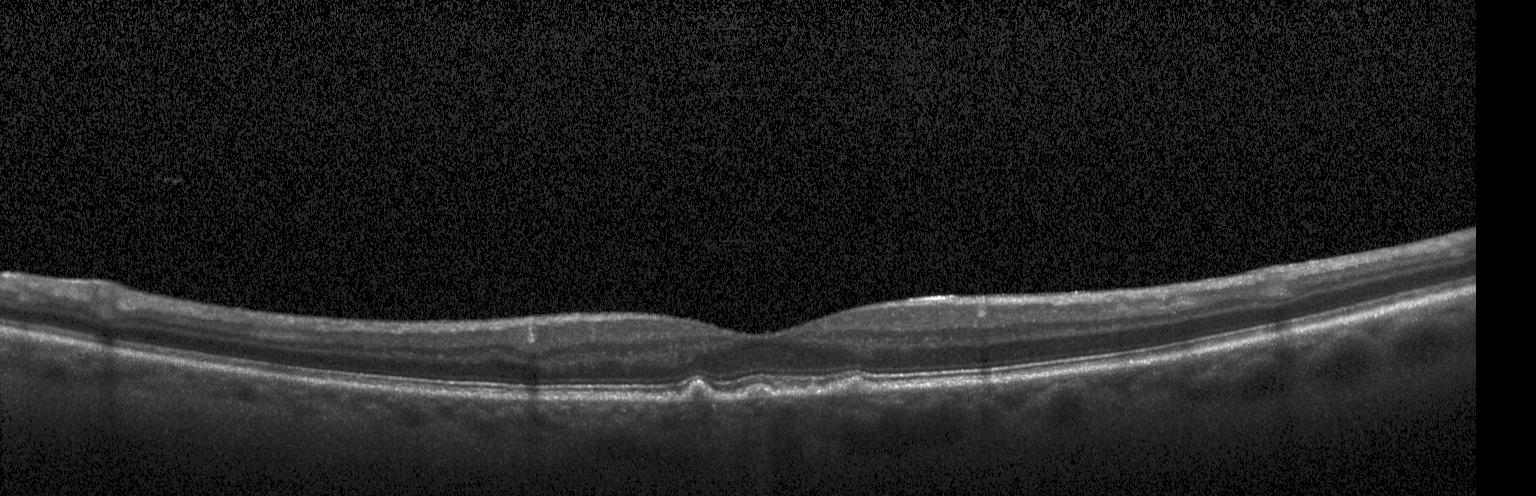

Retinal OCT cross-section · through the macula · instrument: Heidelberg Spectralis · SD-OCT.
Dx: multiple drusen.